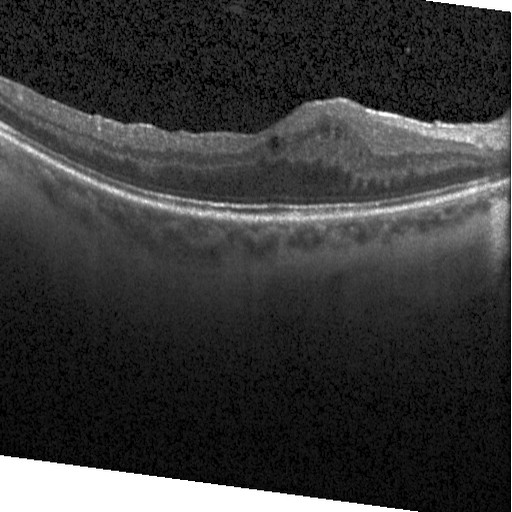 Retinal OCT cross-section, spectral-domain optical coherence tomography.
Diabetic macular edema (DME).